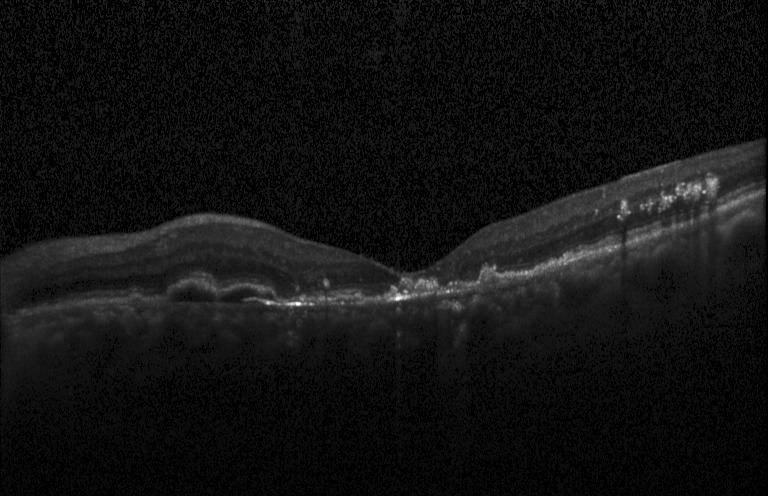

OCT B-scan, centered on the fovea — A choroidal neovascular membrane.